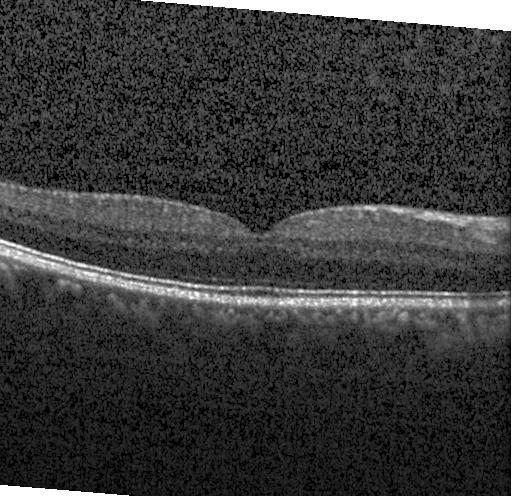 Diagnosis: no choroidal neovascularization, no diabetic macular edema, and no drusen.